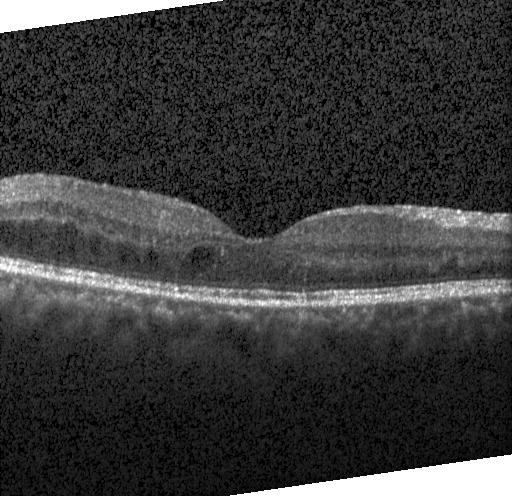
Spectral-domain optical coherence tomography · fovea-centered · instrument: Heidelberg Spectralis · optical coherence tomography B-scan.
Impression: diabetic macular edema.